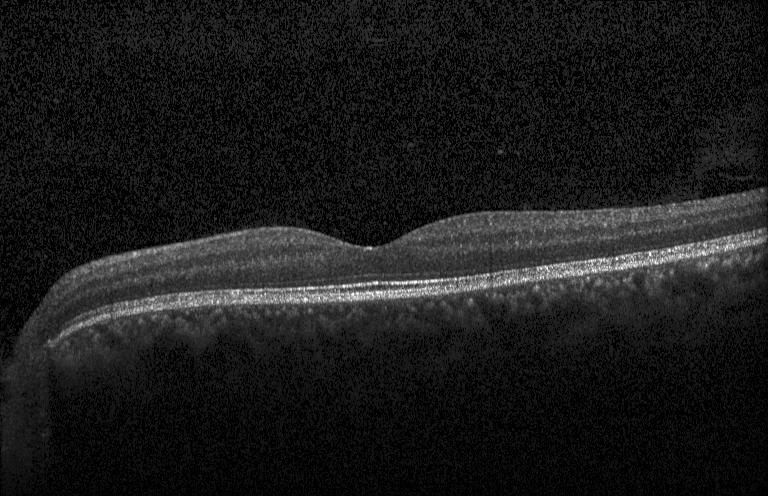

Through the macula · spectral-domain optical coherence tomography · retinal OCT B-scan — Impression: no choroidal neovascularization, no diabetic macular edema, and no drusen.